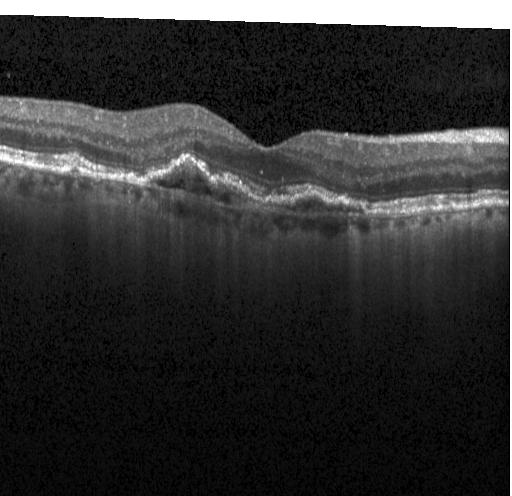
Optical coherence tomography B-scan · fovea-centered — Impression: a choroidal neovascular membrane.